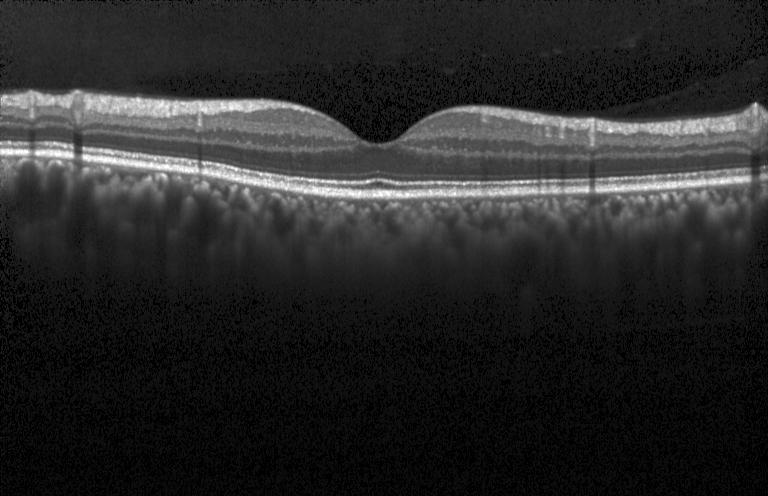 Spectral-domain OCT B-scan: no CNV, DME, or drusen.